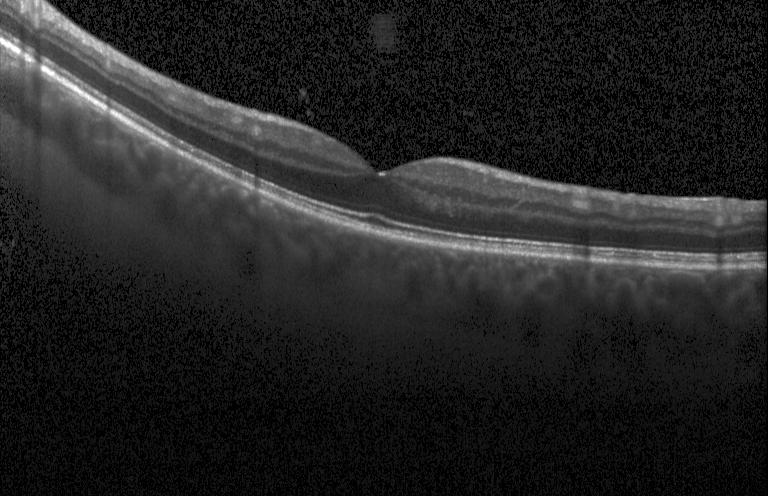
OCT B-scan showing no evidence of choroidal neovascularization, diabetic macular edema, or drusen.